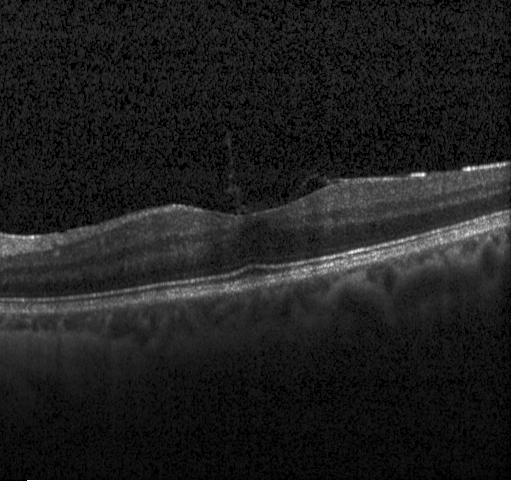

OCT finding: no CNV, DME, or drusen.